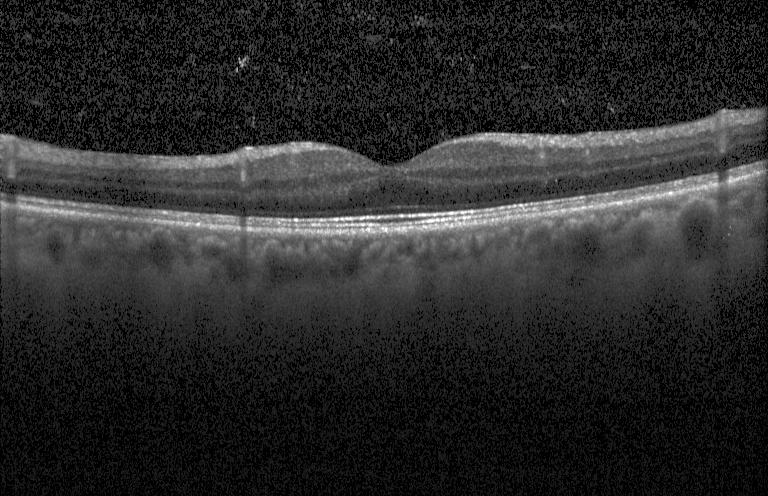

Retinal OCT cross-section.
Impression: neither choroidal neovascularization, diabetic macular edema, nor drusen.